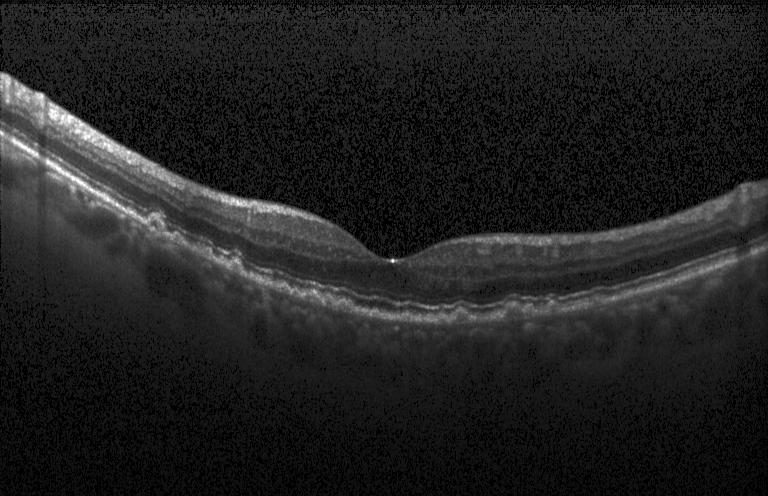 Retinal OCT B-scan — Diagnosis: sub-RPE drusenoid deposits.